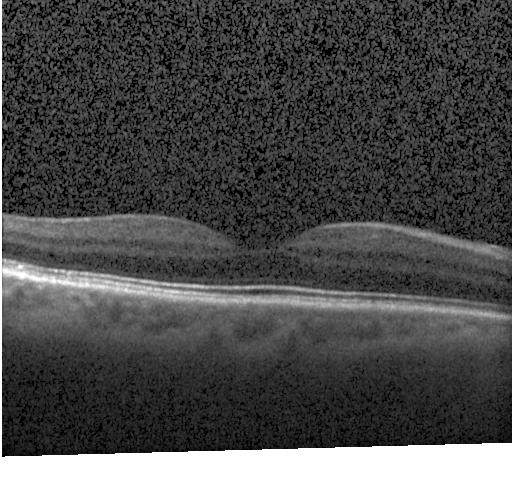 Macular OCT demonstrating no choroidal neovascularization, diabetic macular edema, or drusen.